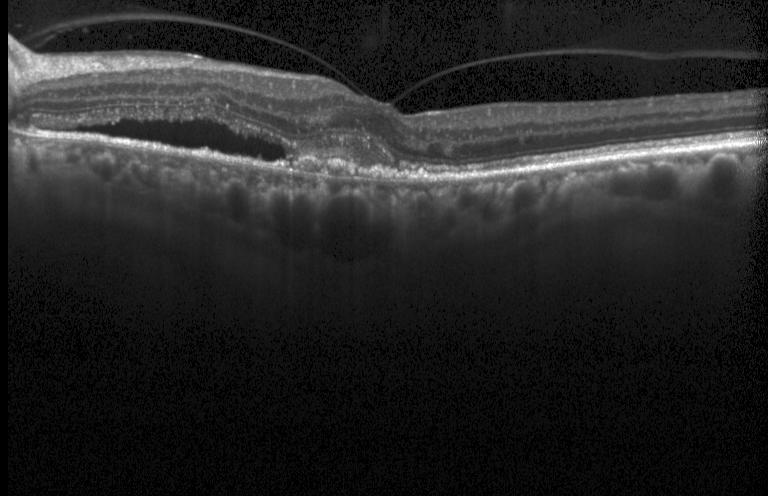 Retinal OCT cross-section · macular scan. The scan shows a choroidal neovascular membrane.